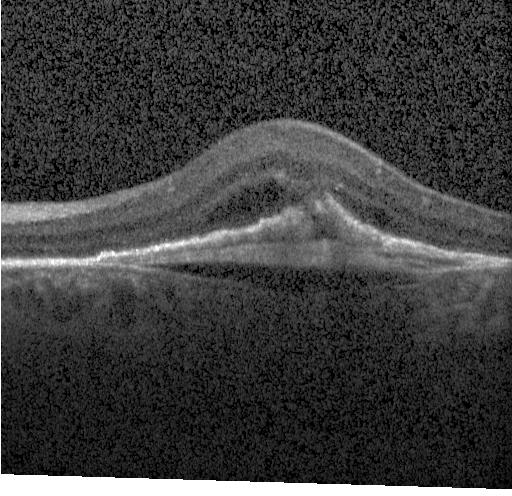
Instrument: Heidelberg Spectralis; retinal OCT cross-section.
The scan shows a choroidal neovascular membrane.